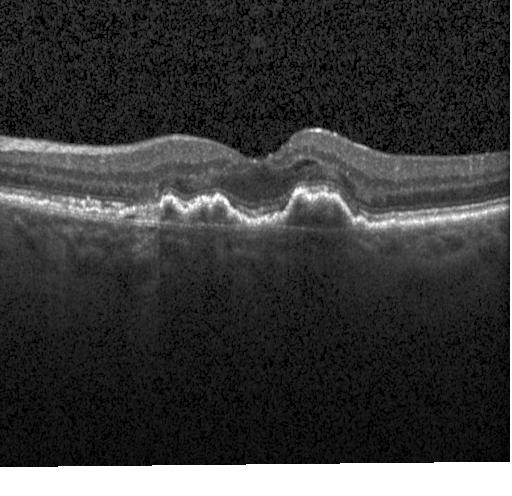

OCT B-scan · fovea-centered — Diagnosis: a choroidal neovascular membrane.